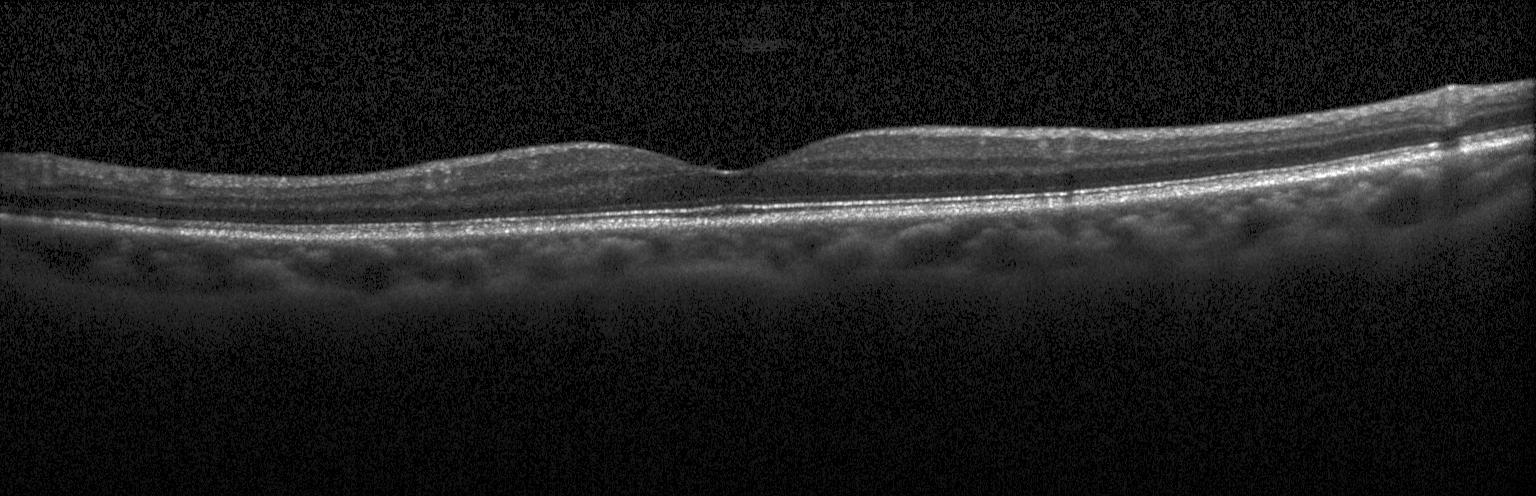
No CNV, DME, or drusen.